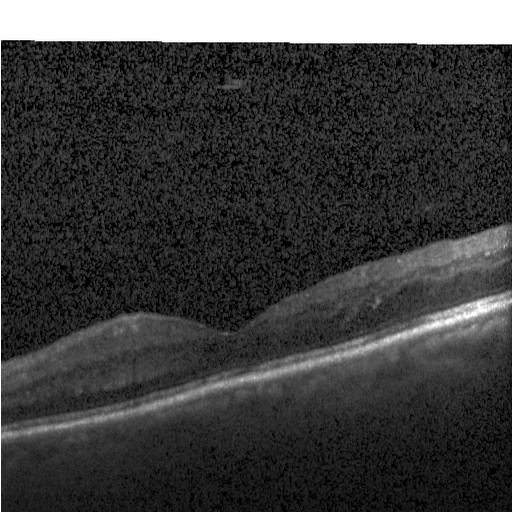

OCT B-scan.
Diagnosis: diabetic macular edema.